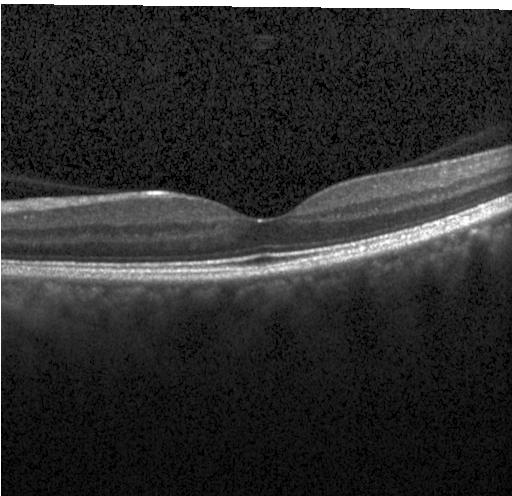

OCT B-scan — Diagnosis: no evidence of choroidal neovascularization, diabetic macular edema, or drusen.